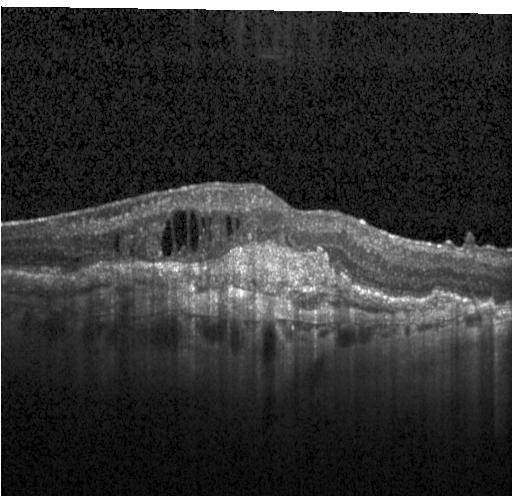 OCT finding: a choroidal neovascular membrane.